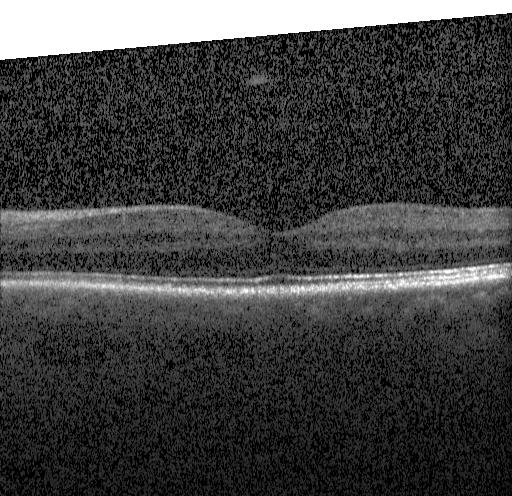

Retinal OCT cross-section showing no CNV, no DME, and no drusen.